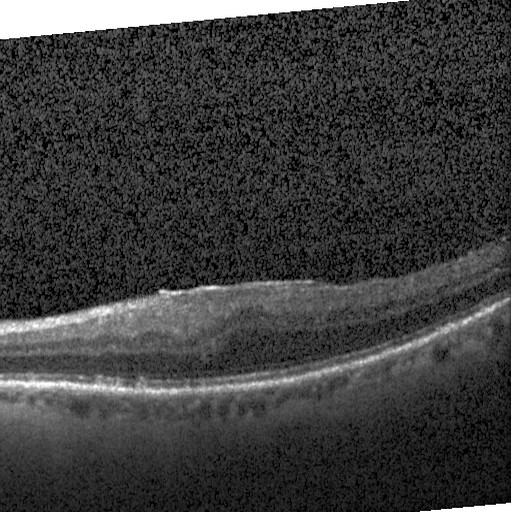 Dx: DME.